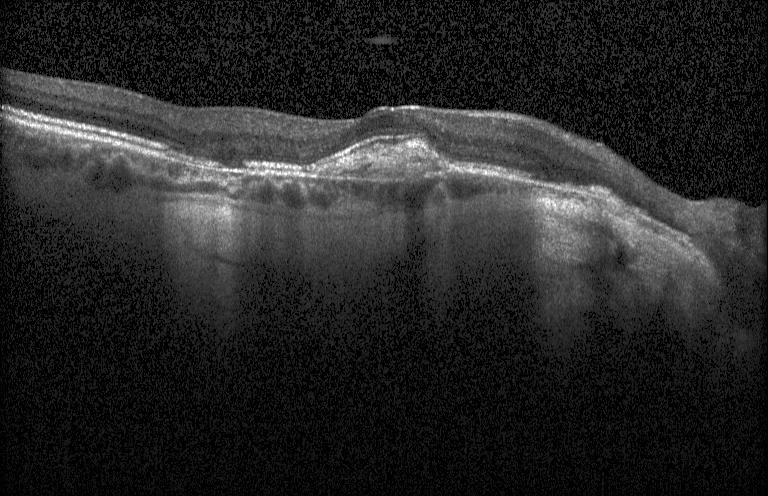

Optical coherence tomography scan — A choroidal neovascular membrane.